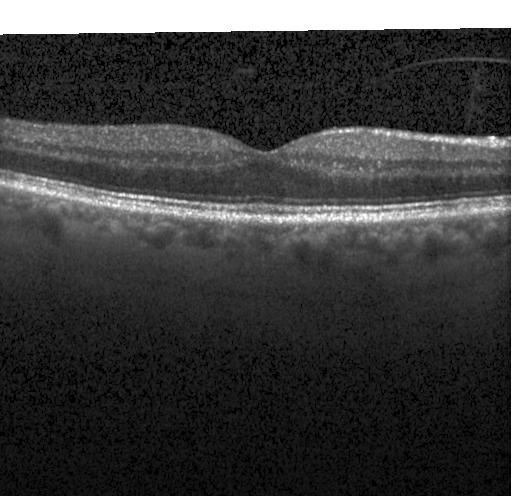 OCT B-scan showing no CNV, DME, or drusen.